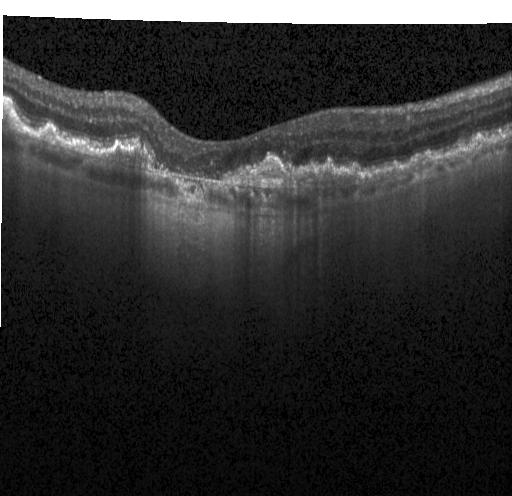 Retinal OCT B-scan
Finding: choroidal neovascularization (CNV).